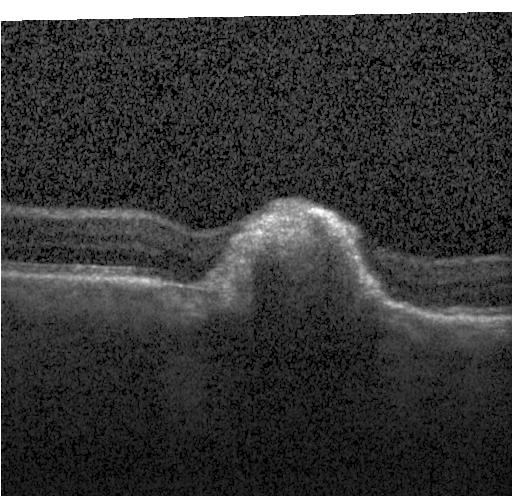 Retinal OCT cross-section
Dx: a choroidal neovascular membrane.